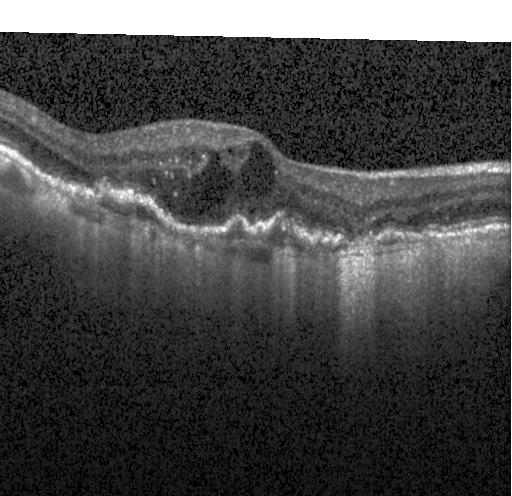 OCT line scan.
Macular OCT: CNV.